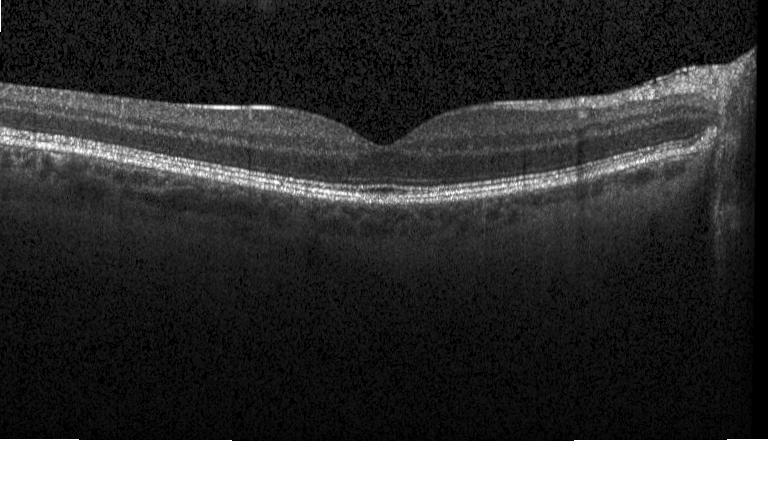
Diagnosis: no choroidal neovascularization, diabetic macular edema, or drusen.